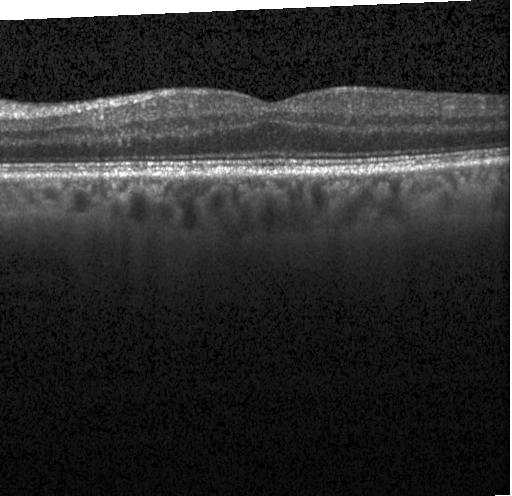 Retinal OCT cross-section; through the macula
No evidence of choroidal neovascularization, diabetic macular edema, or drusen.